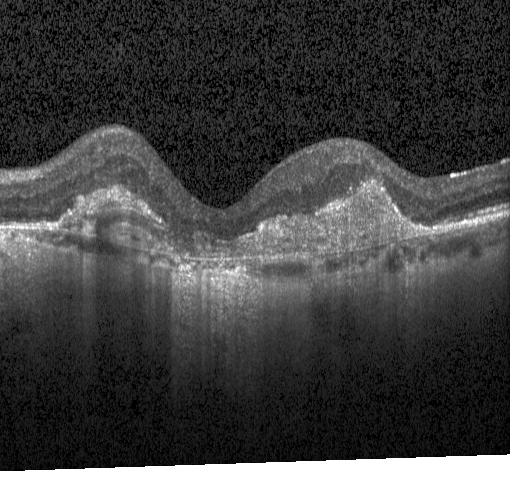 Diagnosis: choroidal neovascularization.